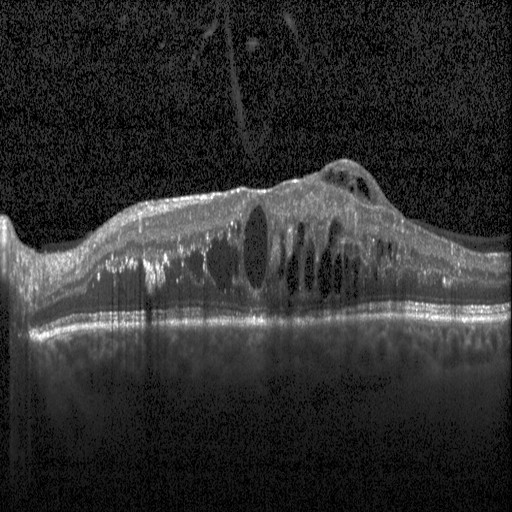

OCT finding: DME.